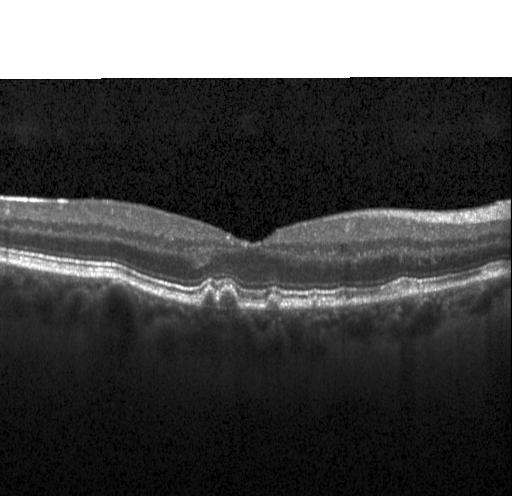 Retinal OCT B-scan · spectral-domain optical coherence tomography · Heidelberg Spectralis OCT system — The scan shows multiple drusen.